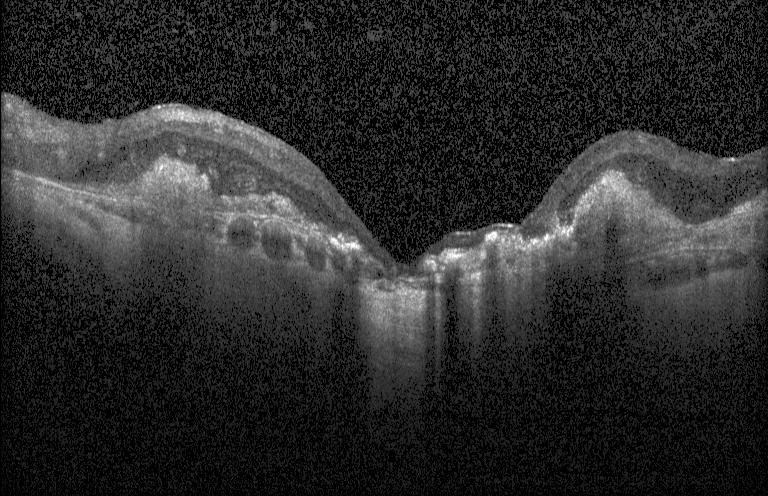

Retinal OCT B-scan
A choroidal neovascular membrane.